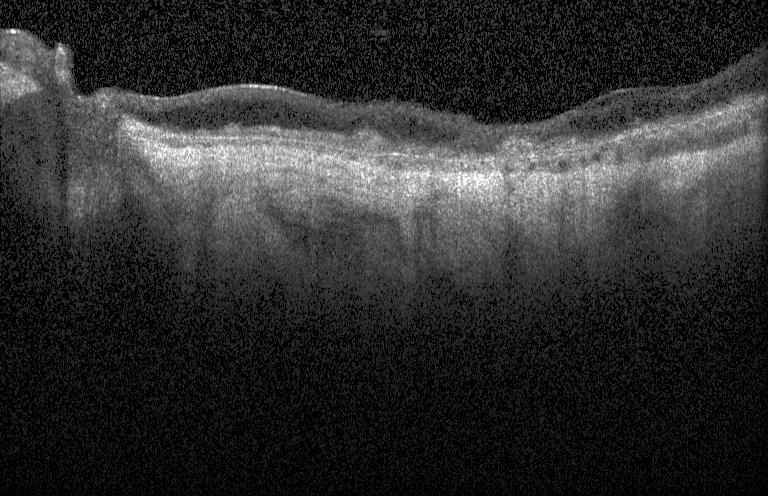
SD-OCT; macular scan; OCT line scan; acquired on a Heidelberg Spectralis.
OCT finding: choroidal neovascularization (CNV).